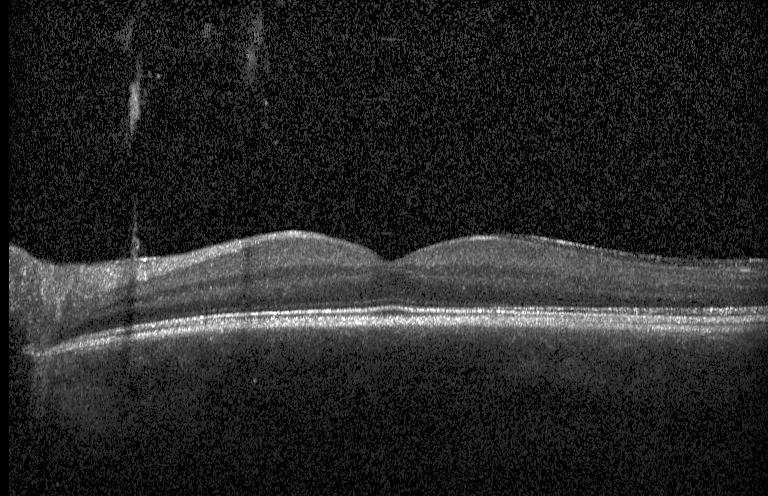 Retinal OCT B-scan · spectral-domain OCT · instrument: Heidelberg Spectralis — Impression: neither choroidal neovascularization, diabetic macular edema, nor drusen.